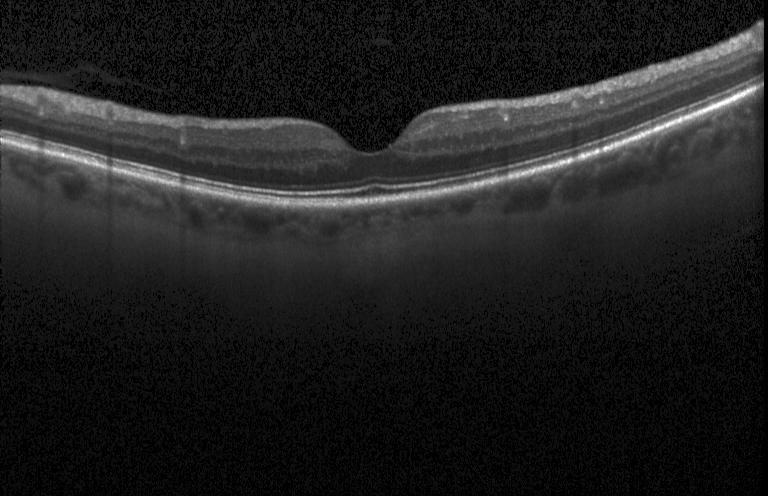
The scan shows no choroidal neovascularization, no diabetic macular edema, and no drusen.